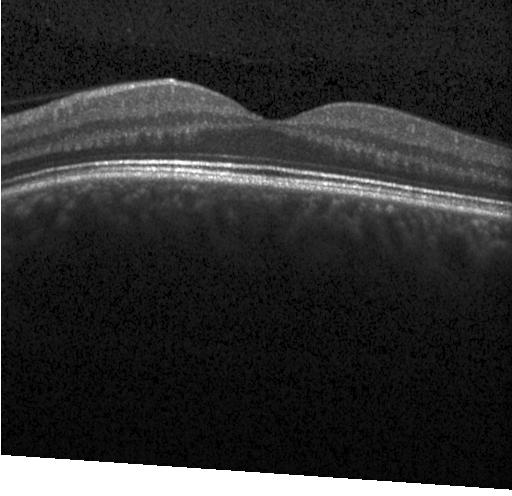

Spectral-domain OCT B-scan: neither choroidal neovascularization, diabetic macular edema, nor drusen.